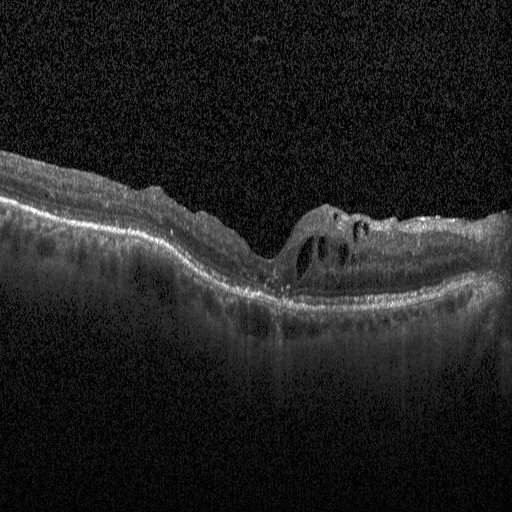

Macular scan, OCT line scan
Diagnosis: DME.